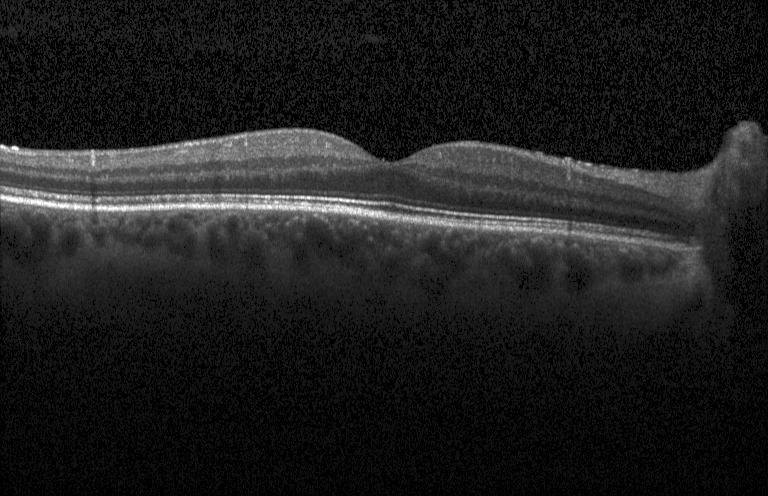 Fovea-centered; optical coherence tomography scan; acquired on a Heidelberg Spectralis; spectral-domain OCT
Diagnosis: neither choroidal neovascularization, diabetic macular edema, nor drusen.